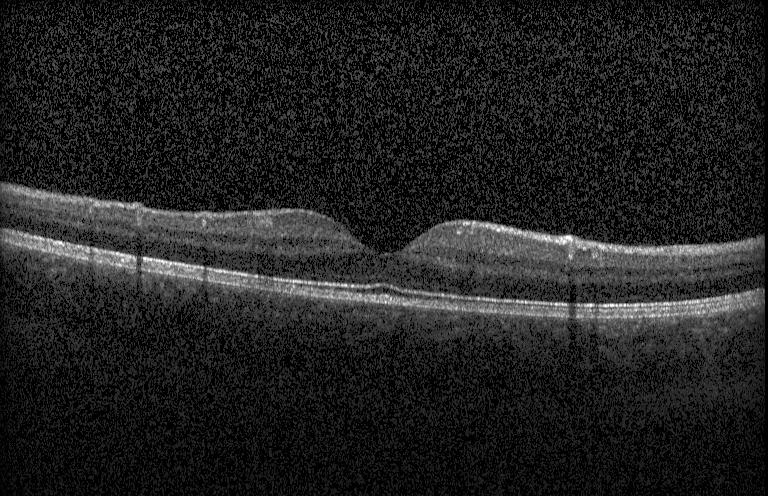
Heidelberg Spectralis OCT system, retinal OCT cross-section — Diagnosis: neither choroidal neovascularization, diabetic macular edema, nor drusen.